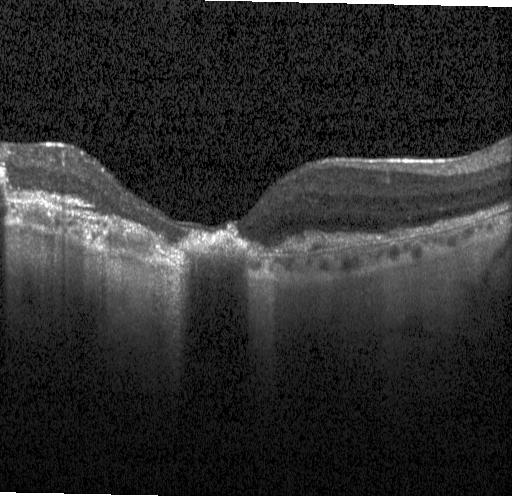 Retinal OCT cross-section showing choroidal neovascularization (CNV).